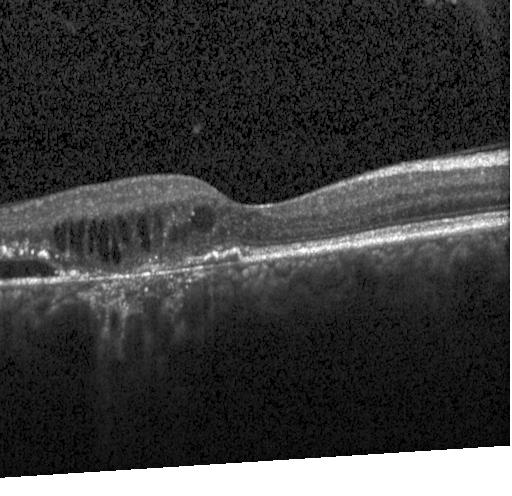

SD-OCT · optical coherence tomography scan — Choroidal neovascularization (CNV).